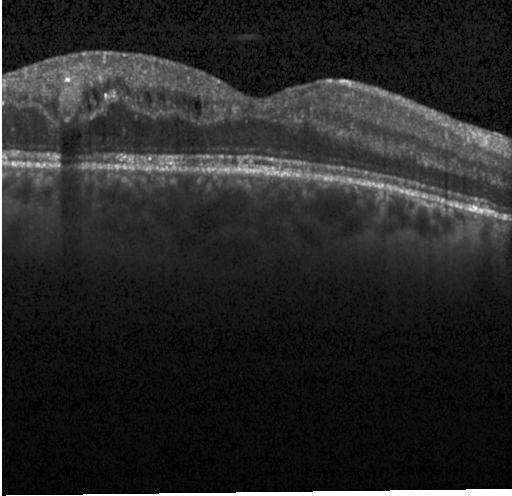
Spectral-domain OCT B-scan: DME.